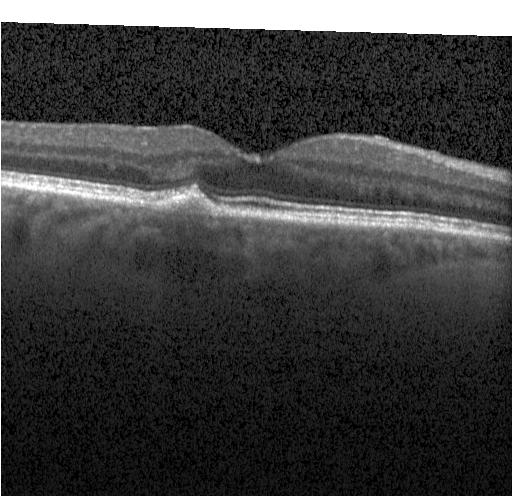

Macular scan · optical coherence tomography scan · instrument: Heidelberg Spectralis. Impression: sub-RPE drusenoid deposits.